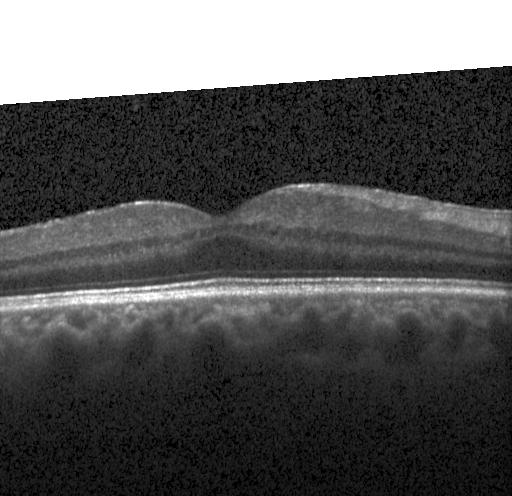
Heidelberg Spectralis, optical coherence tomography B-scan, spectral-domain optical coherence tomography, horizontal scan through the fovea. Assessment: no choroidal neovascularization, diabetic macular edema, or drusen.